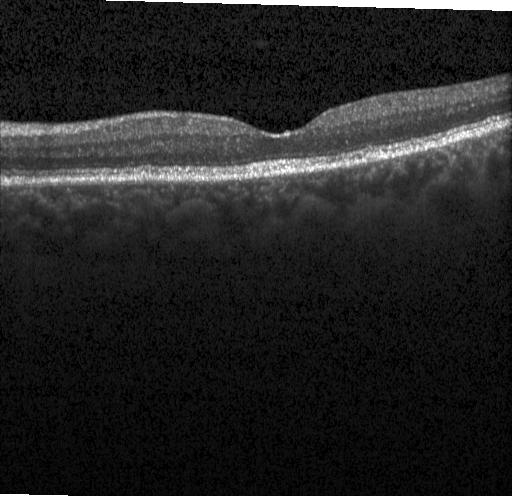 Impression: no choroidal neovascularization, no diabetic macular edema, and no drusen.